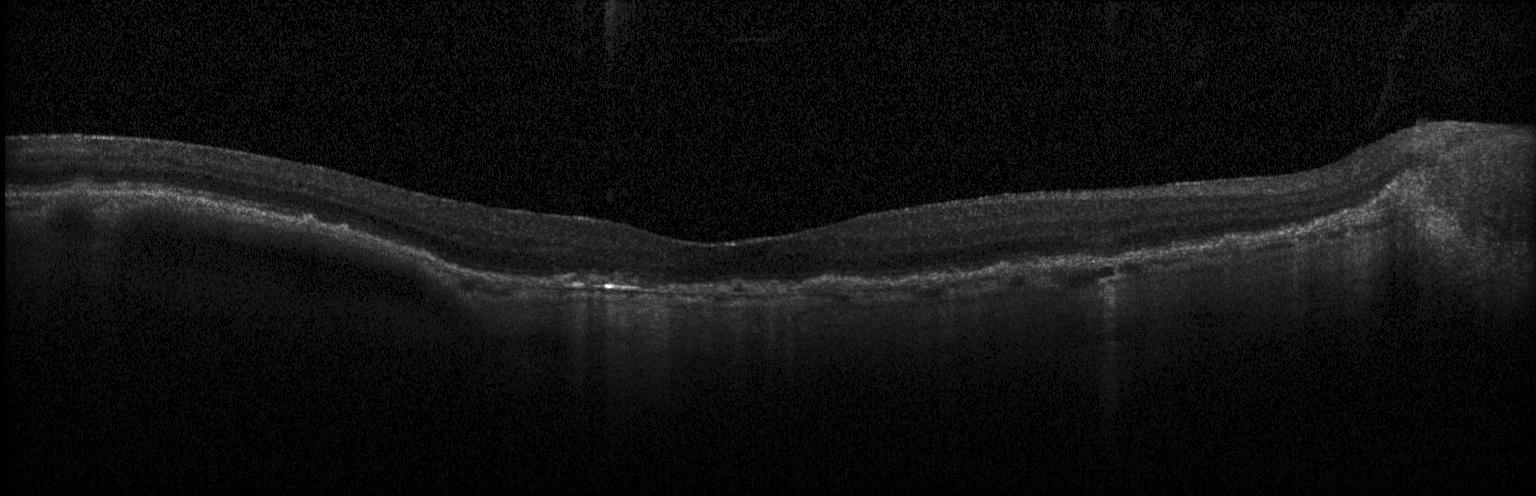 Optical coherence tomography scan · macular scan · instrument: Heidelberg Spectralis. Impression: choroidal neovascularization.